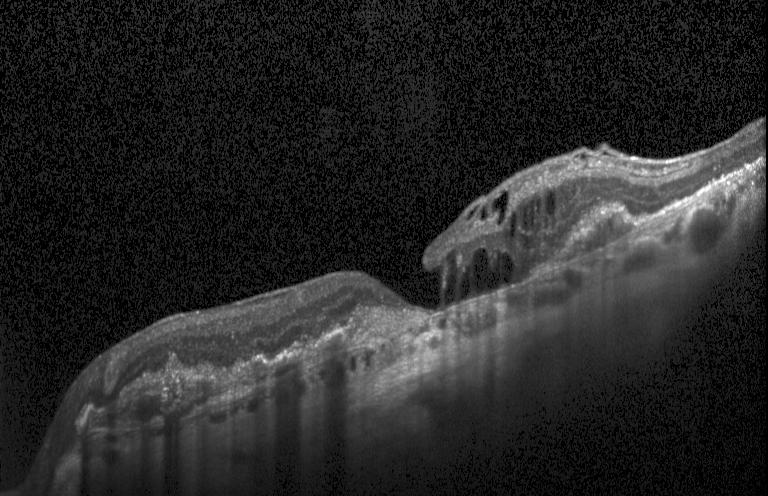 Optical coherence tomography scan · spectral-domain optical coherence tomography.
The scan shows a choroidal neovascular membrane.